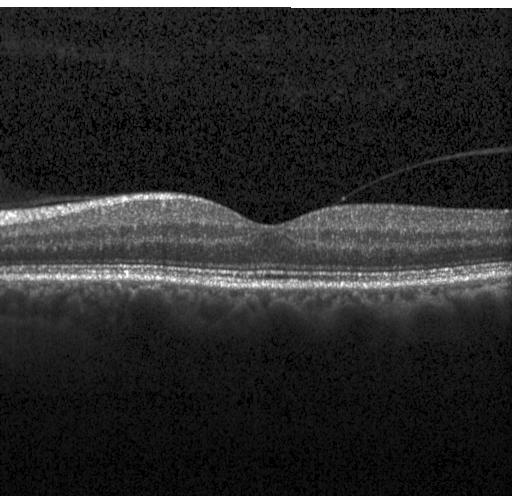
OCT B-scan.
Impression: neither CNV, DME, nor drusen.